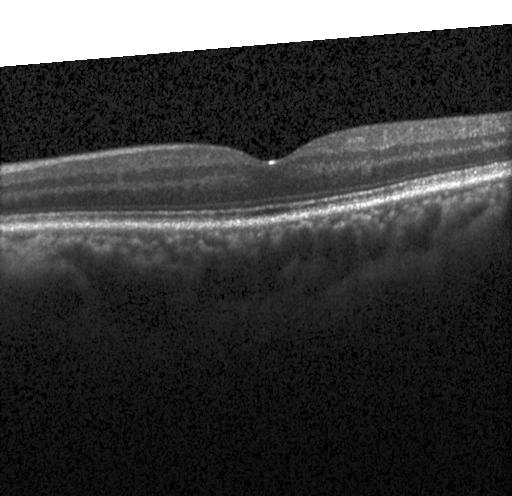

OCT B-scan · Heidelberg Spectralis · centered on the fovea — Finding: no CNV, no DME, and no drusen.